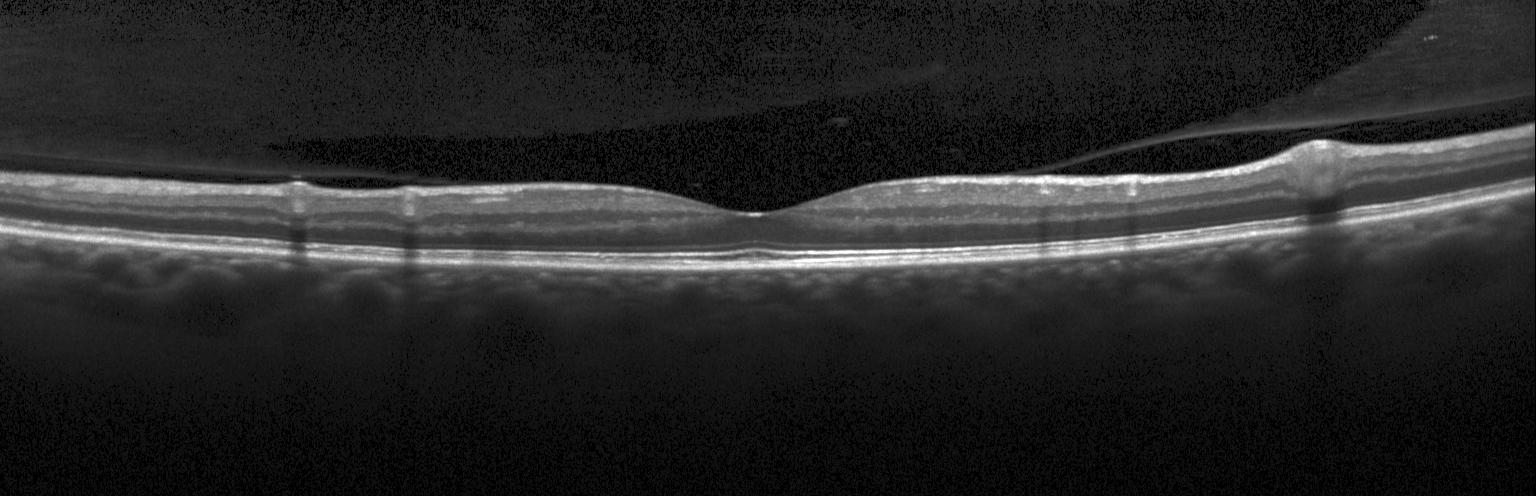 Heidelberg Spectralis OCT system. Optical coherence tomography scan. Spectral-domain optical coherence tomography
Diagnosis: neither choroidal neovascularization, diabetic macular edema, nor drusen.